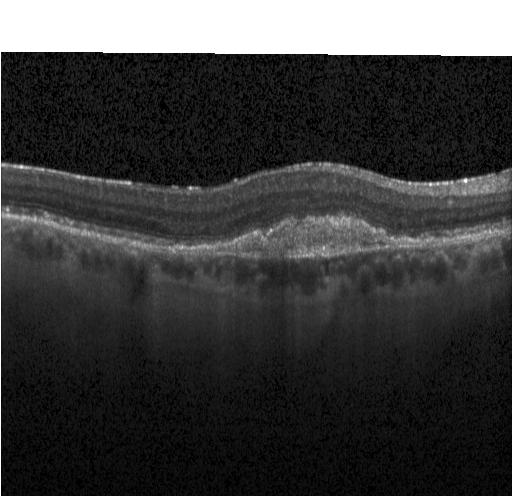 Retinal OCT B-scan. This B-scan demonstrates a choroidal neovascular membrane.